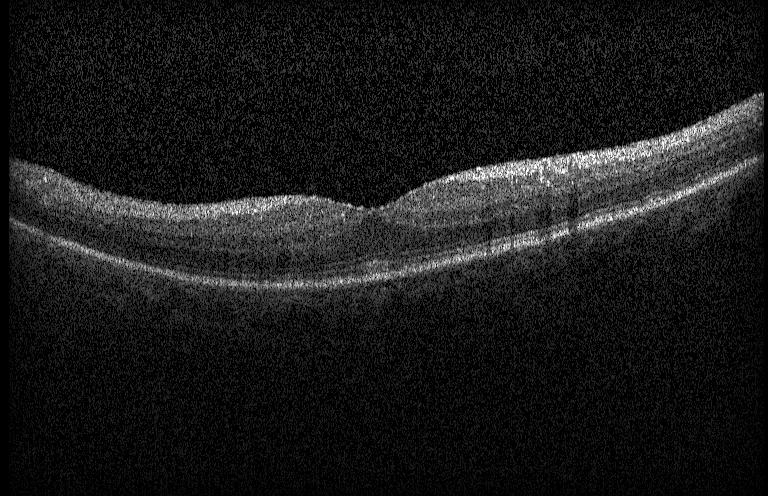
Spectral-domain OCT B-scan: neither choroidal neovascularization, diabetic macular edema, nor drusen.